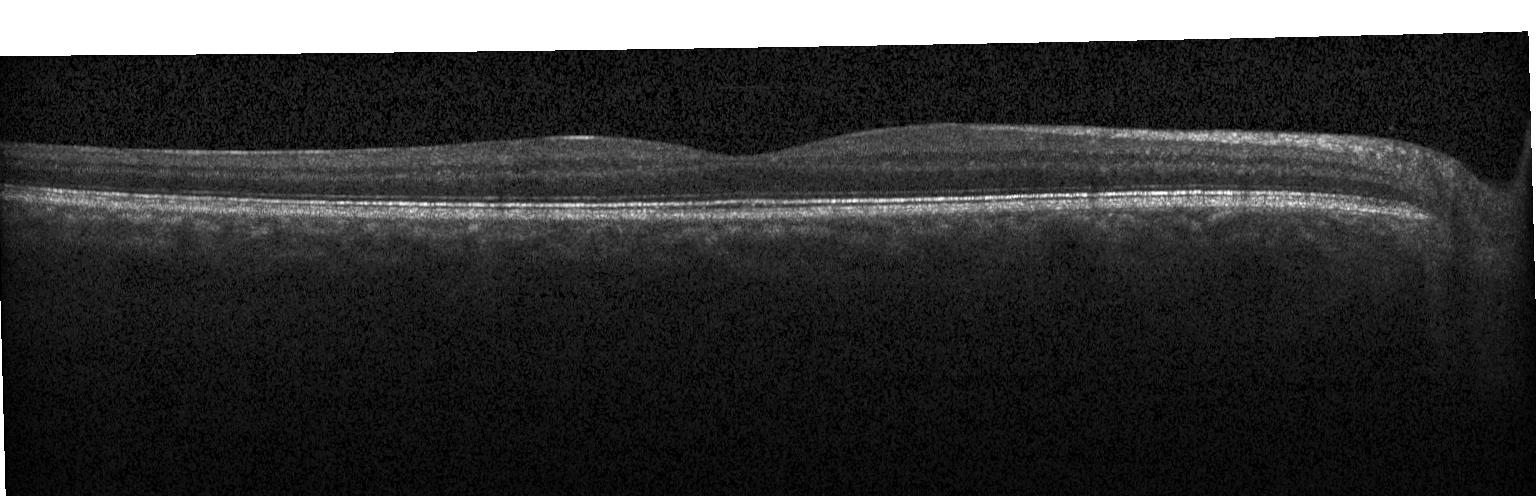

Retinal OCT B-scan.
The scan shows neither CNV, DME, nor drusen.